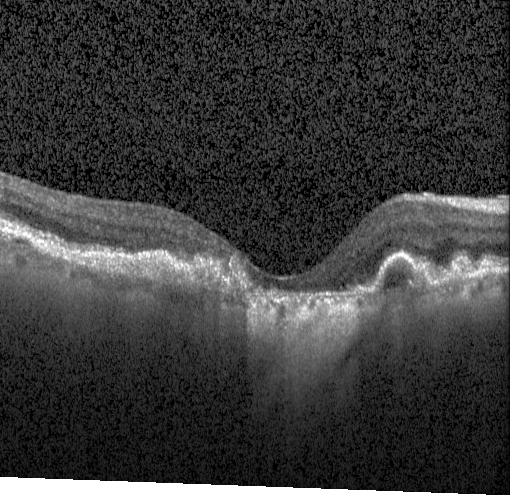
Macular scan, spectral-domain OCT, optical coherence tomography scan
Finding: a choroidal neovascular membrane.